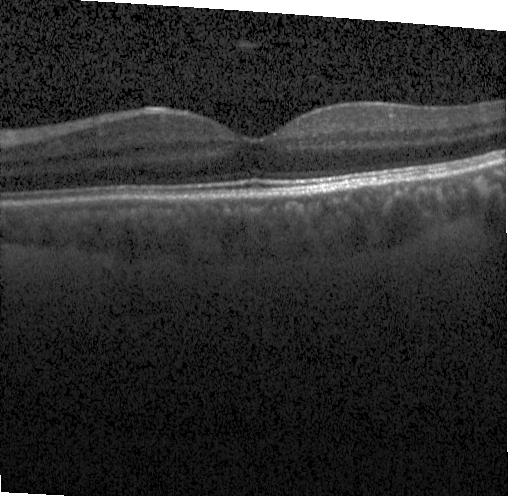

SD-OCT · optical coherence tomography scan · horizontal scan through the fovea · instrument: Heidelberg Spectralis. Dx: no evidence of CNV, DME, or drusen.